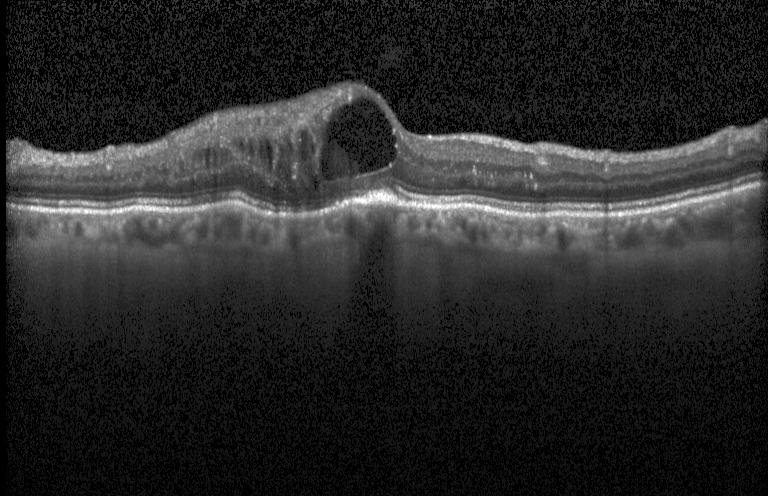
Dx: diabetic macular edema.